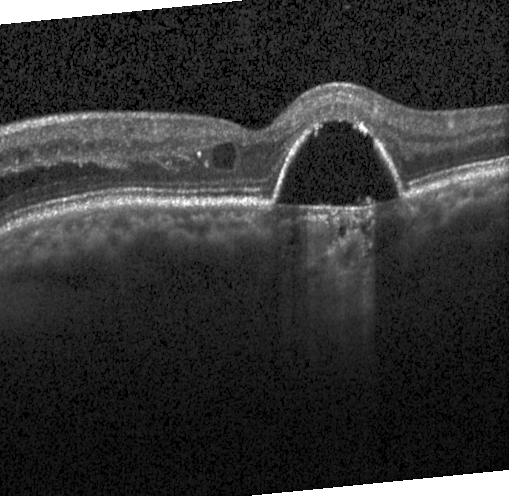
This B-scan demonstrates choroidal neovascularization.